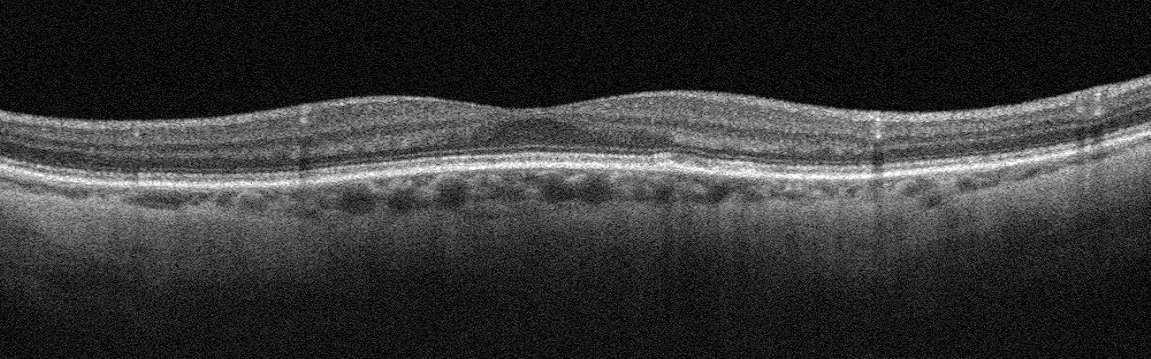

Spectral-domain OCT B-scan: age-related macular degeneration (AMD).